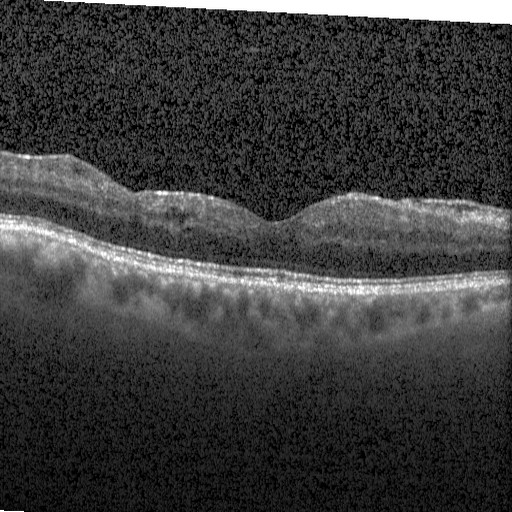

Centered on the fovea. SD-OCT. Heidelberg Spectralis. Optical coherence tomography scan
Finding: diabetic macular edema.